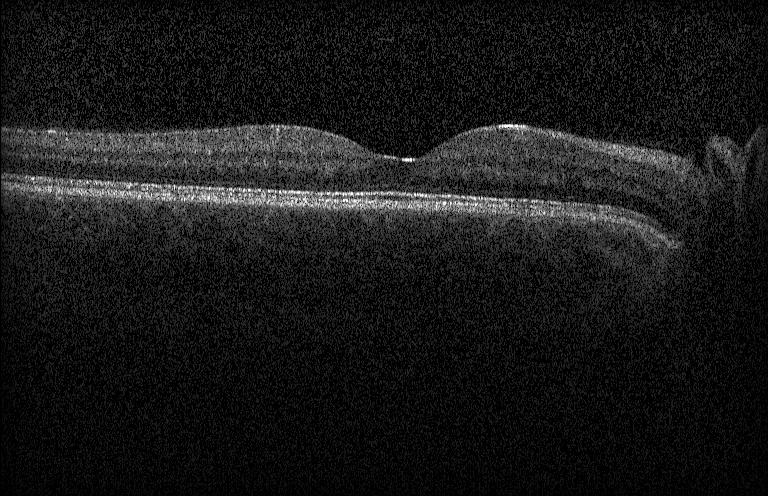
OCT scan showing no choroidal neovascularization, no diabetic macular edema, and no drusen.